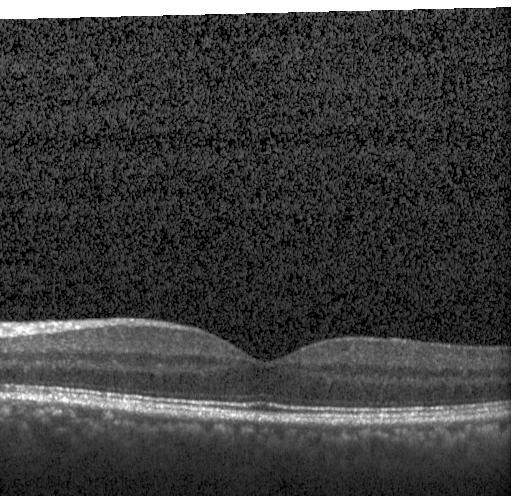

OCT B-scan.
Impression: no choroidal neovascularization, no diabetic macular edema, and no drusen.